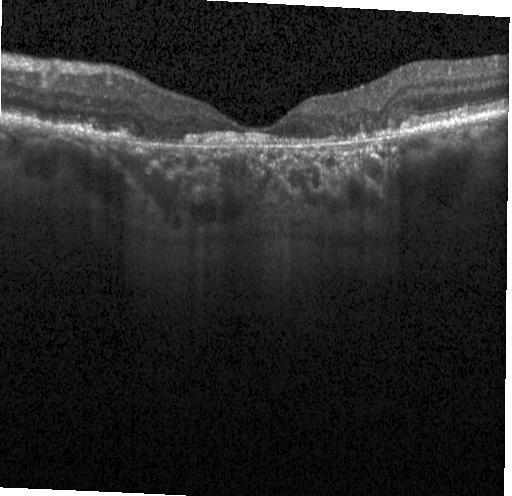 Retinal OCT cross-section showing choroidal neovascularization (CNV).